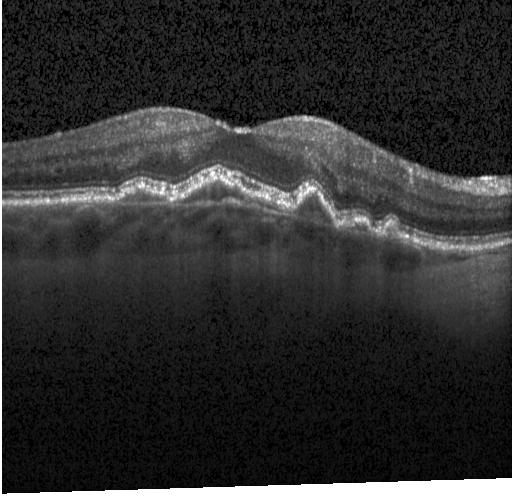

Optical coherence tomography B-scan. Spectral-domain OCT. Heidelberg Spectralis OCT system. Fovea-centered
Diagnosis: a choroidal neovascular membrane.